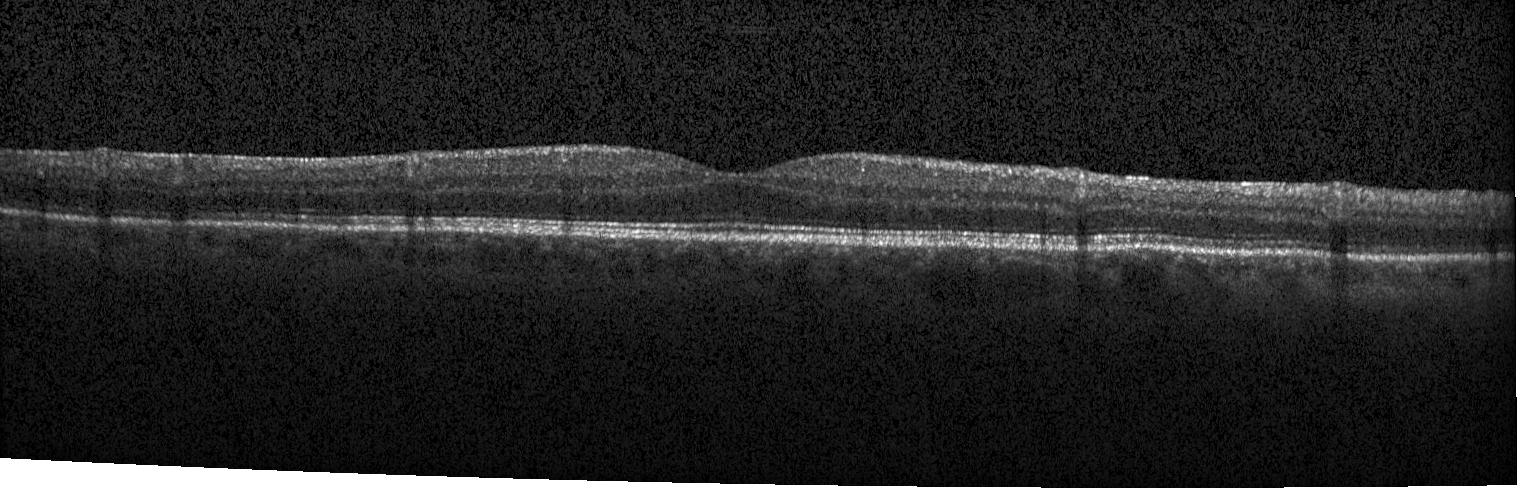
OCT finding: no CNV, DME, or drusen.